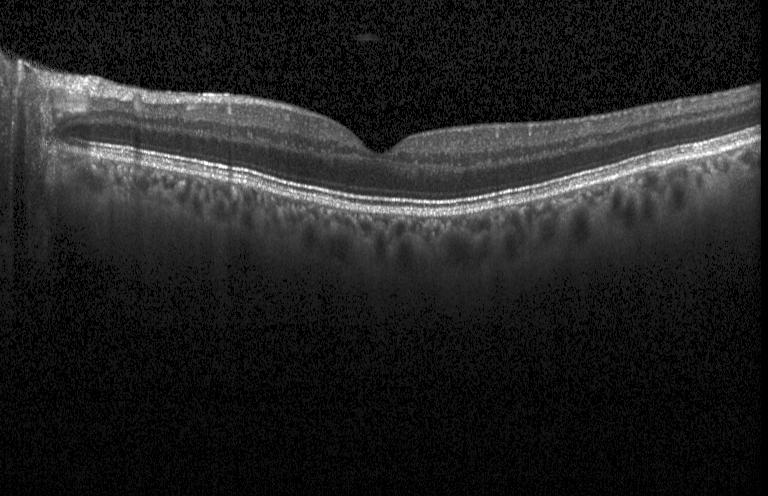

OCT line scan. Diagnosis: no choroidal neovascularization, no diabetic macular edema, and no drusen.